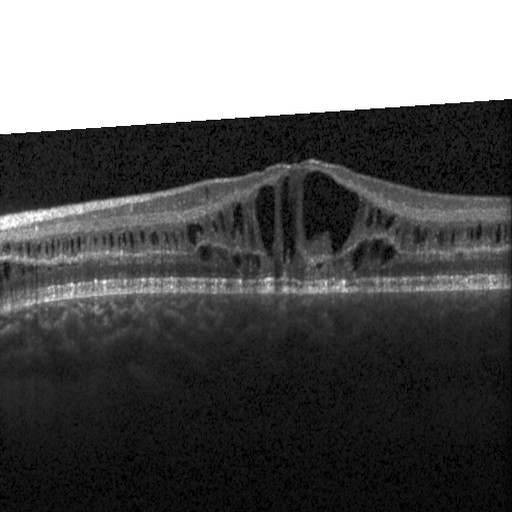

OCT finding: diabetic macular edema.